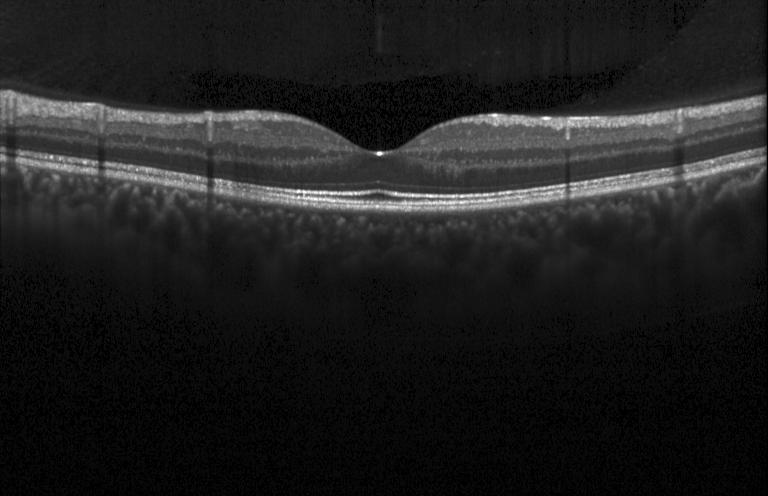 Retinal OCT B-scan.
OCT finding: neither CNV, DME, nor drusen.